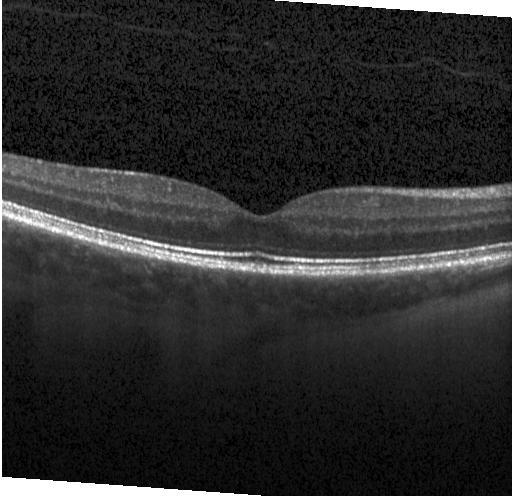 Diagnosis: no evidence of choroidal neovascularization, diabetic macular edema, or drusen.